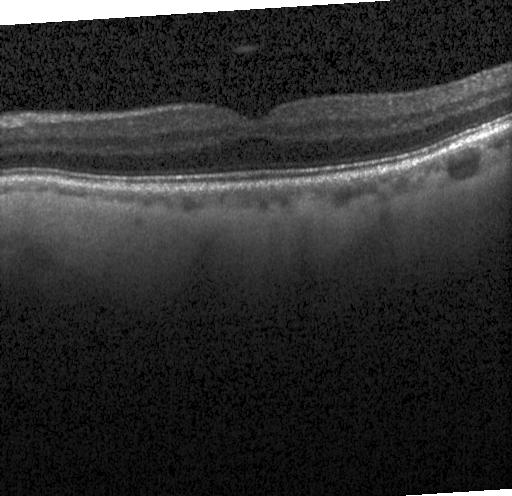
Centered on the fovea, spectral-domain OCT, OCT line scan, acquired on a Heidelberg Spectralis. Diagnosis: no choroidal neovascularization, diabetic macular edema, or drusen.